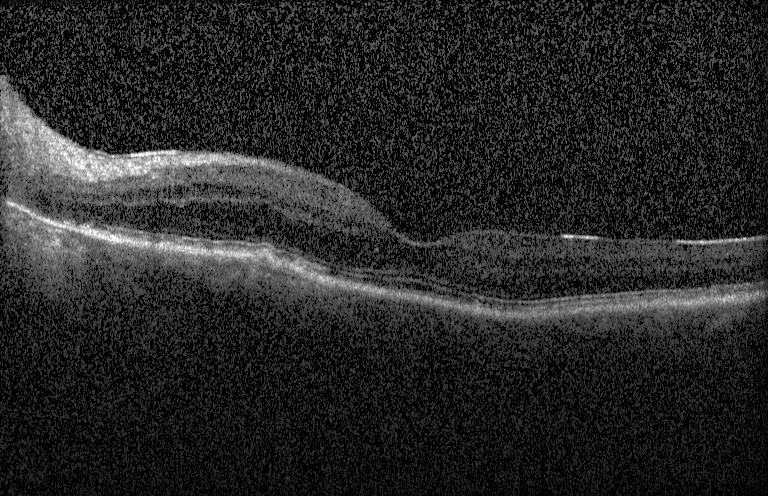
Acquired on a Heidelberg Spectralis · OCT B-scan.
Finding: drusen.